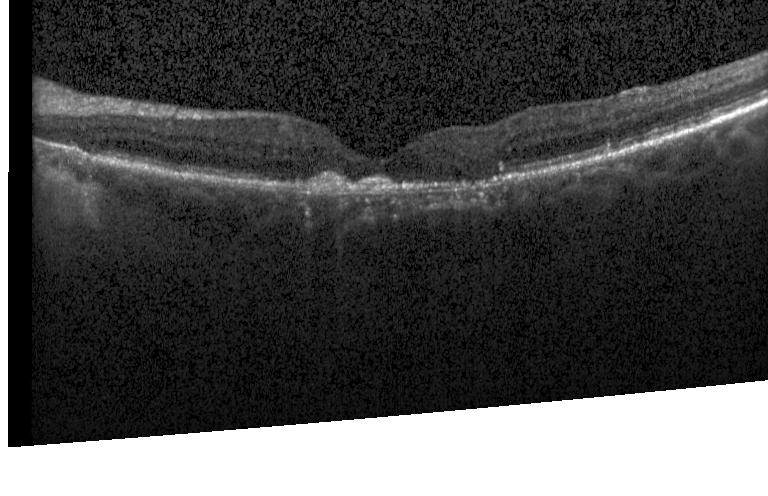

OCT finding: a choroidal neovascular membrane.